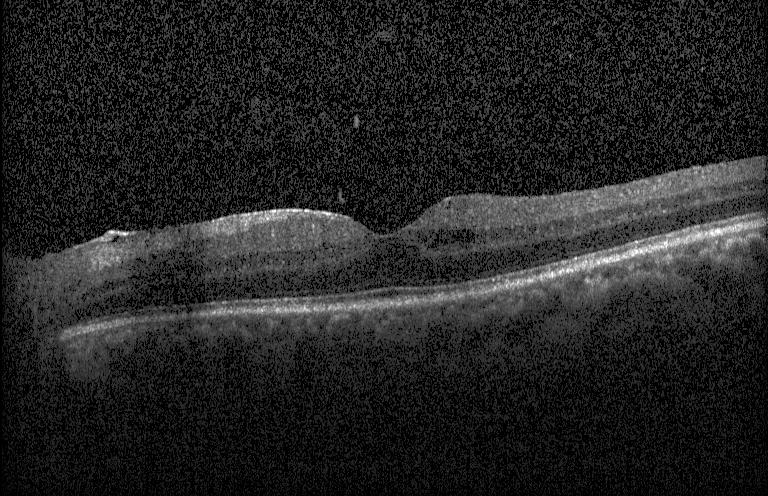 Horizontal scan through the fovea · Heidelberg Spectralis OCT system · retinal OCT B-scan. Impression: DME.